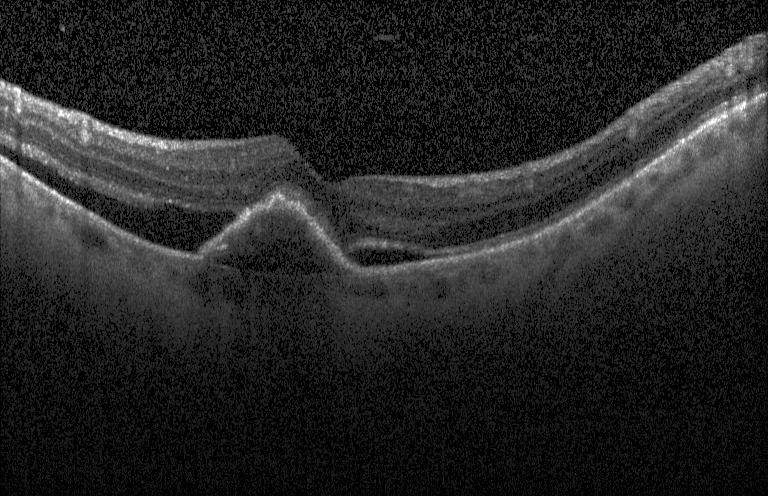
Choroidal neovascularization (CNV).